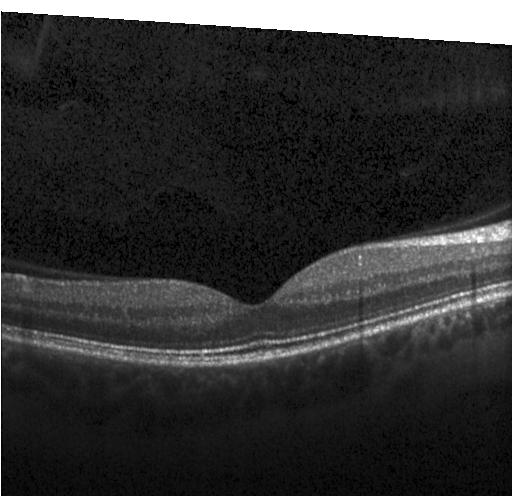
Spectral-domain OCT; optical coherence tomography B-scan; fovea-centered. Finding: no choroidal neovascularization, diabetic macular edema, or drusen.